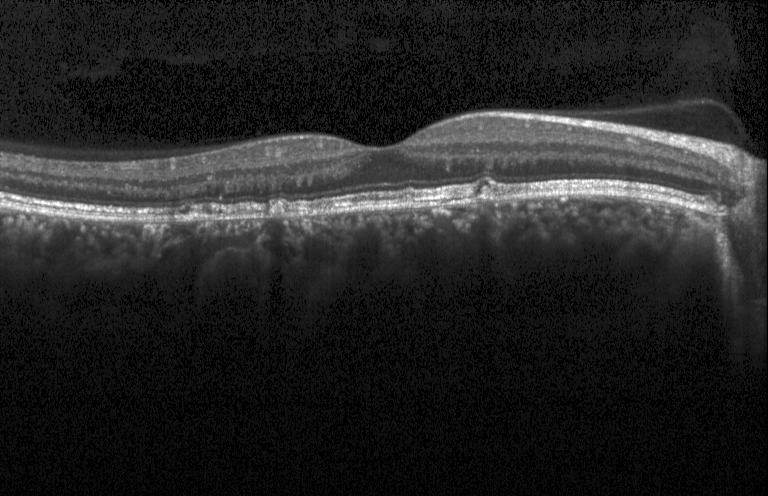

Retinal OCT B-scan
Multiple drusen.